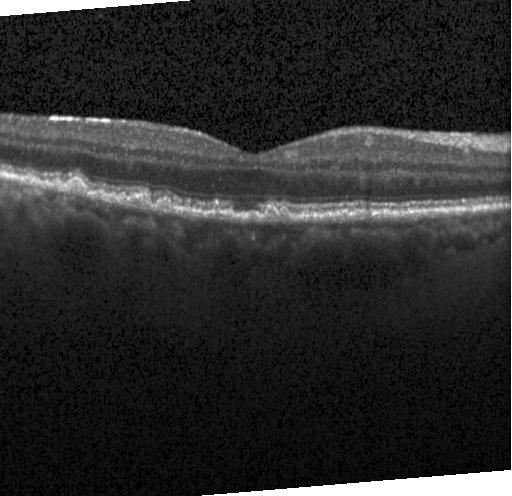

Impression: drusen.